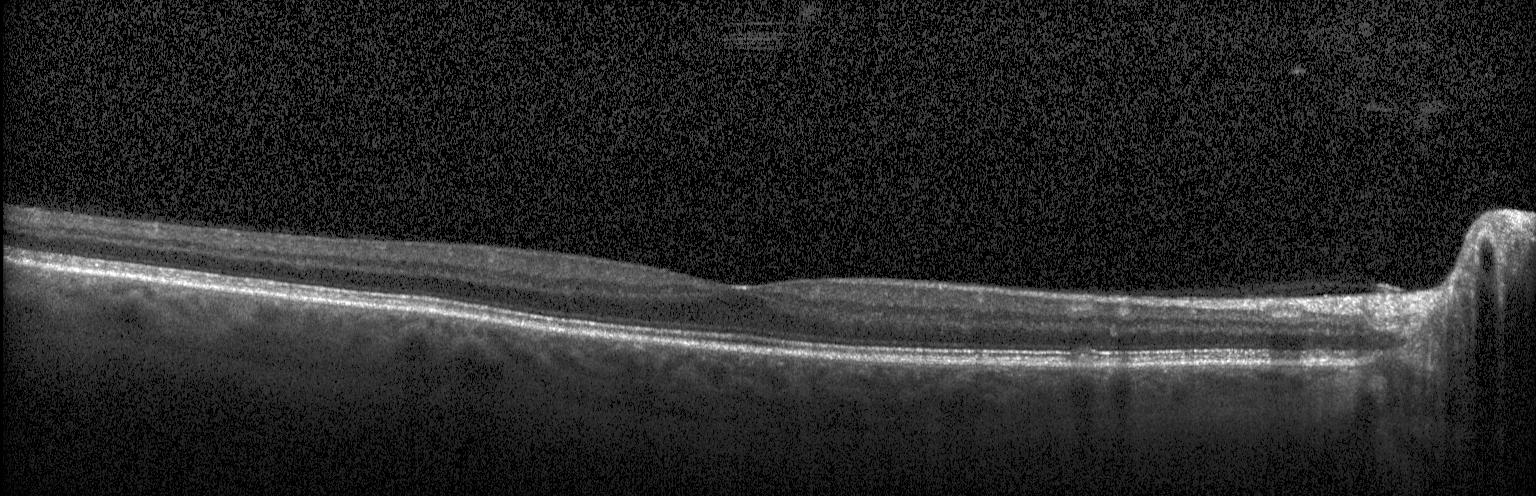
OCT B-scan; horizontal scan through the fovea; SD-OCT; Heidelberg Spectralis
Finding: no CNV, no DME, and no drusen.